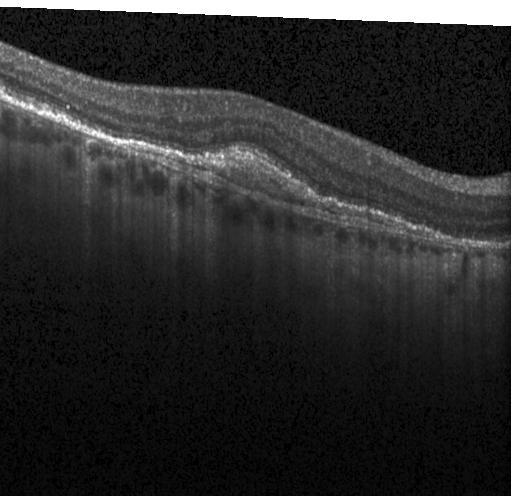 Optical coherence tomography scan.
Impression: CNV.